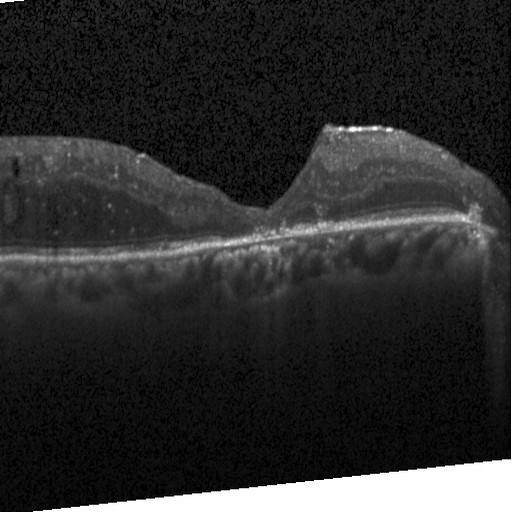 Optical coherence tomography scan. This B-scan demonstrates DME.